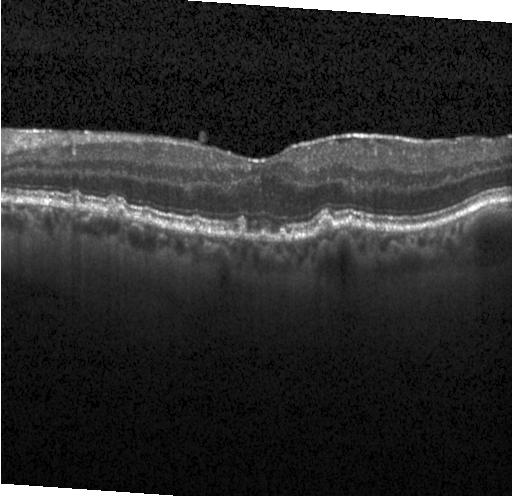

Instrument: Heidelberg Spectralis, retinal OCT cross-section
Macular OCT: sub-RPE drusenoid deposits.